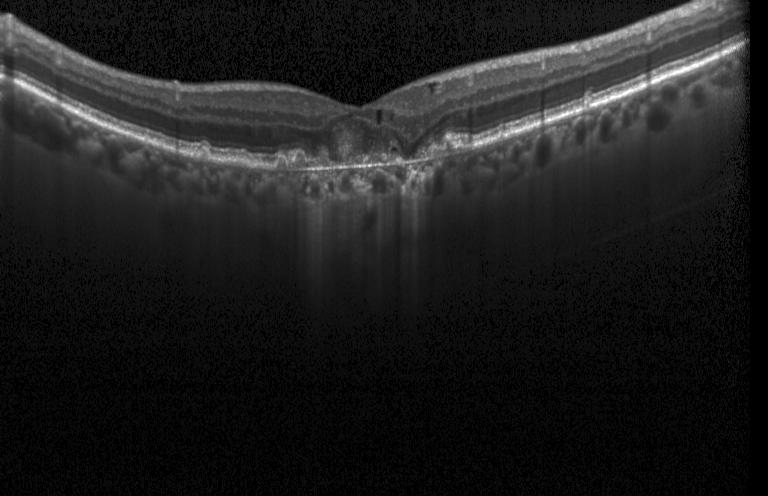 OCT scan showing a choroidal neovascular membrane.